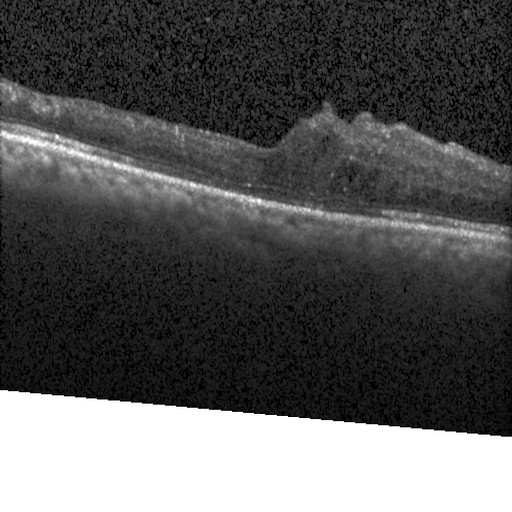 OCT finding: DME.